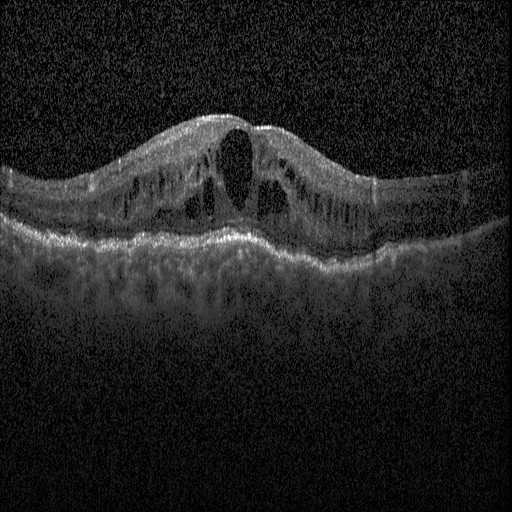 Spectral-domain OCT B-scan: diabetic macular edema (DME).